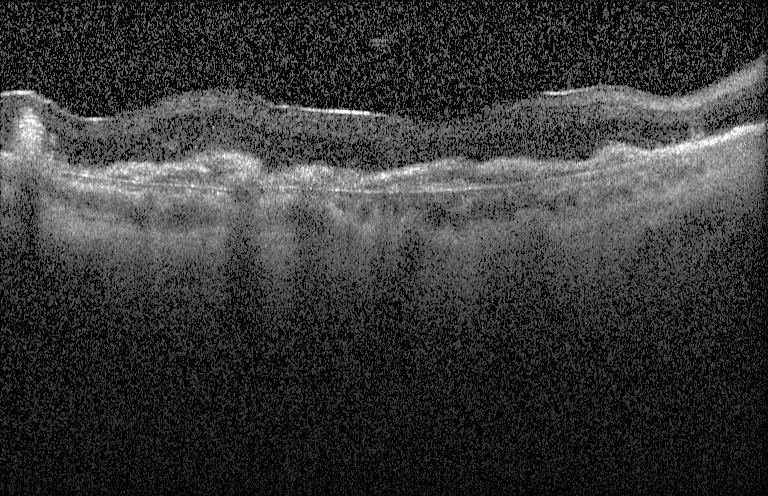 Assessment: choroidal neovascularization (CNV).